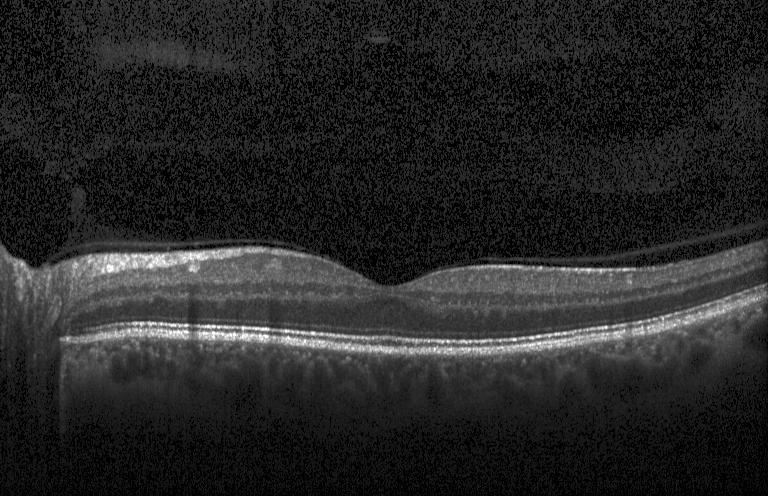 SD-OCT. Retinal OCT B-scan
Macular OCT: no CNV, no DME, and no drusen.